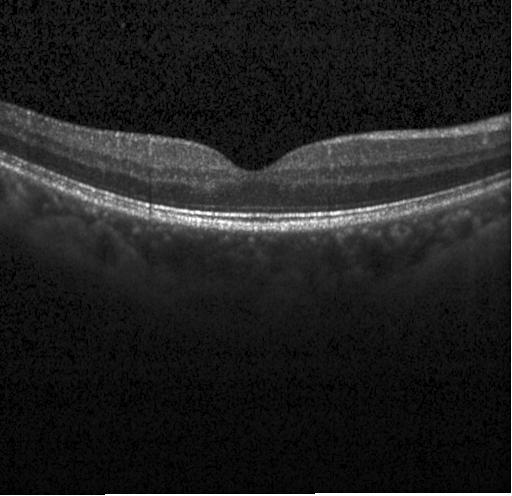 Optical coherence tomography B-scan, Heidelberg Spectralis OCT system, macular scan — This B-scan demonstrates no evidence of choroidal neovascularization, diabetic macular edema, or drusen.